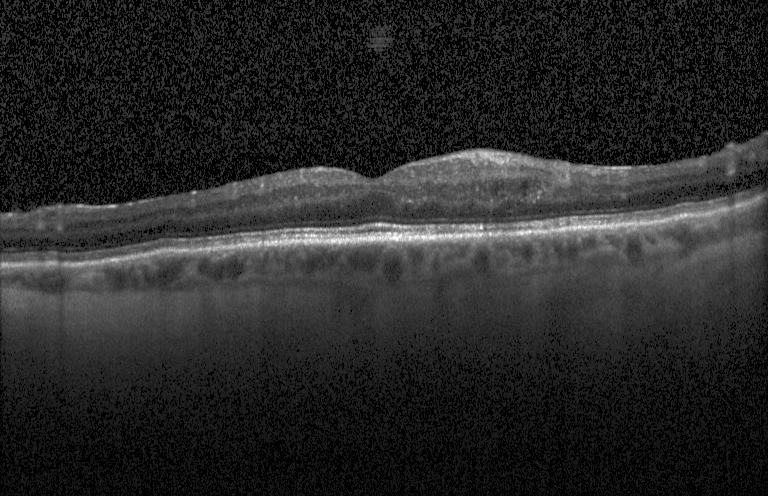
Retinal OCT B-scan. Centered on the fovea. Spectral-domain optical coherence tomography. Instrument: Heidelberg Spectralis.
Impression: diabetic macular edema.